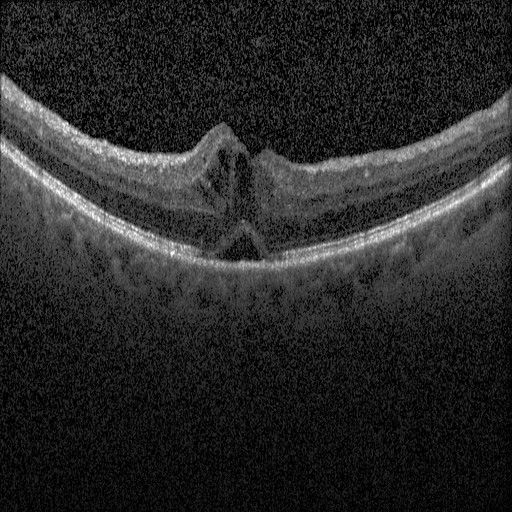 Macular OCT: DME.